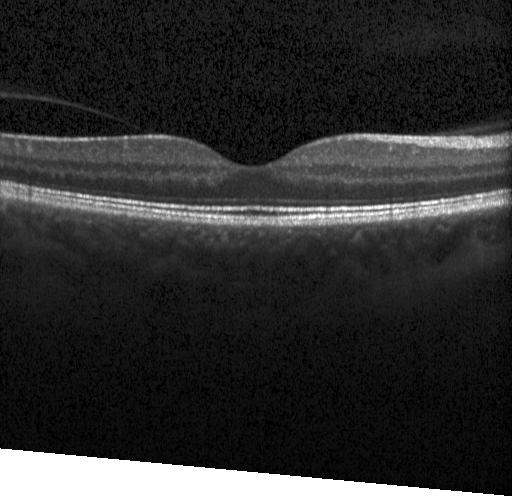
Macular OCT demonstrating neither choroidal neovascularization, diabetic macular edema, nor drusen.